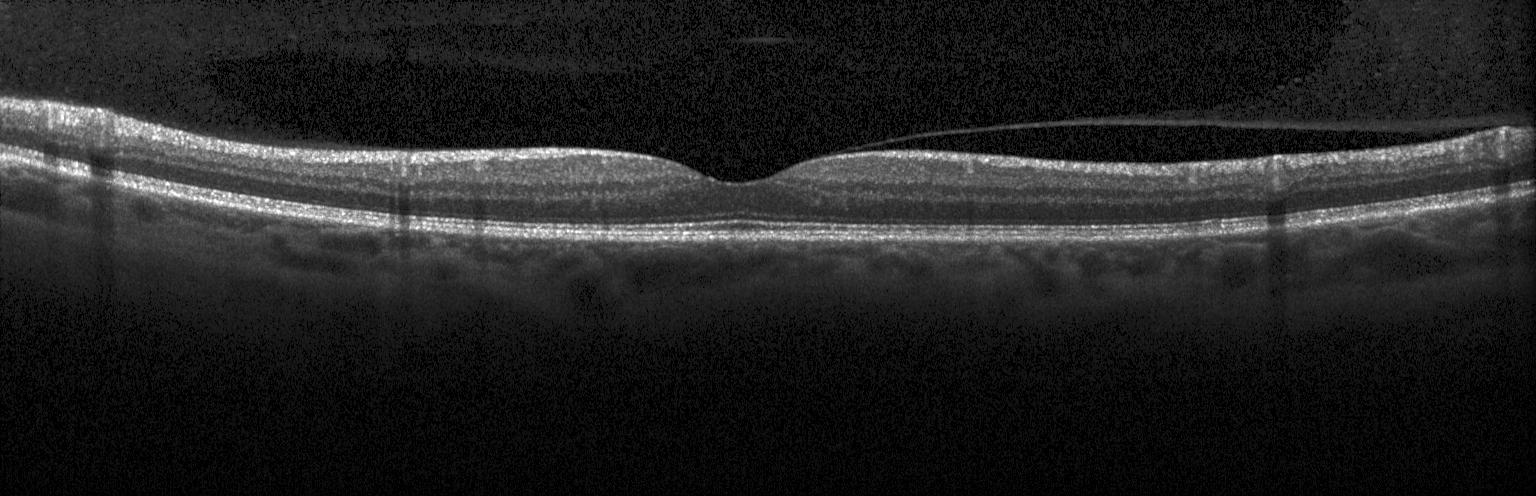 Heidelberg Spectralis; spectral-domain OCT; fovea-centered; optical coherence tomography B-scan — Impression: no evidence of choroidal neovascularization, diabetic macular edema, or drusen.